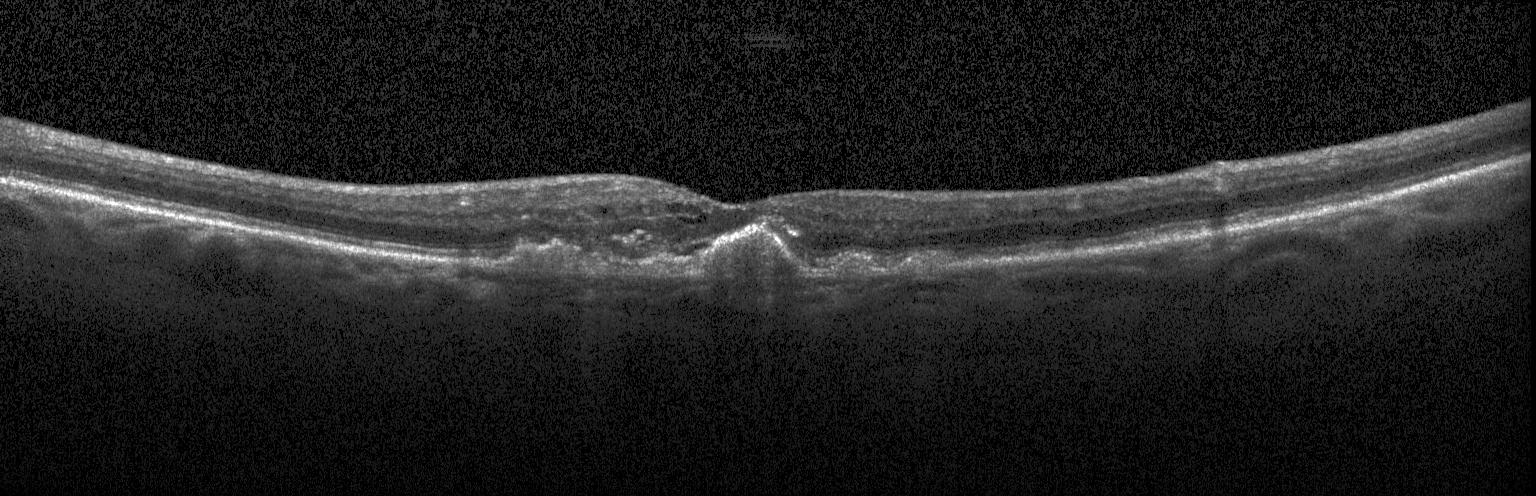 Optical coherence tomography B-scan · Heidelberg Spectralis OCT system · fovea-centered · SD-OCT — Diagnosis: CNV.